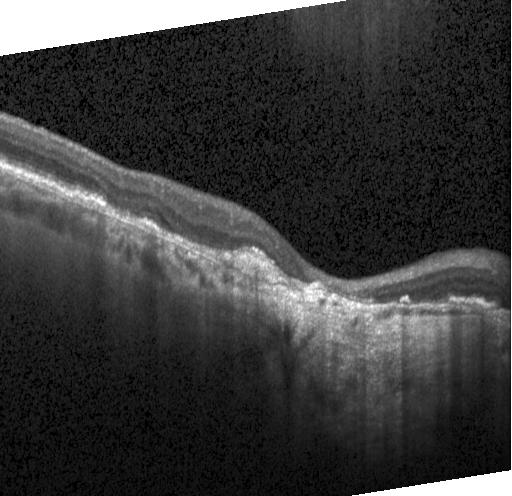
OCT line scan; SD-OCT. The scan shows choroidal neovascularization (CNV).